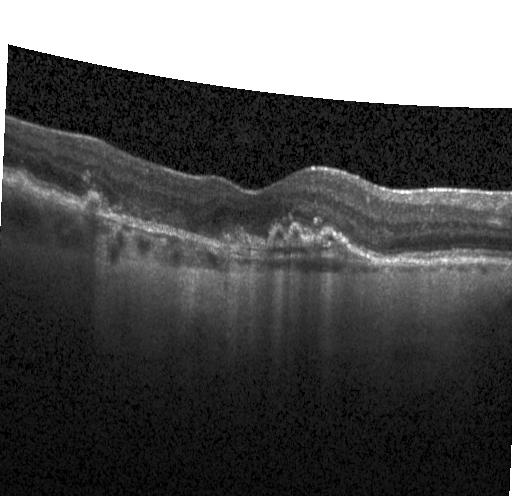
Optical coherence tomography B-scan, spectral-domain optical coherence tomography.
OCT finding: choroidal neovascularization.